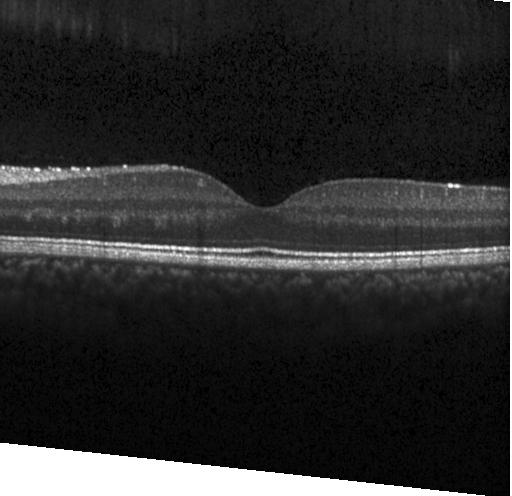 Heidelberg Spectralis, SD-OCT, optical coherence tomography B-scan, macular scan.
OCT finding: no CNV, DME, or drusen.